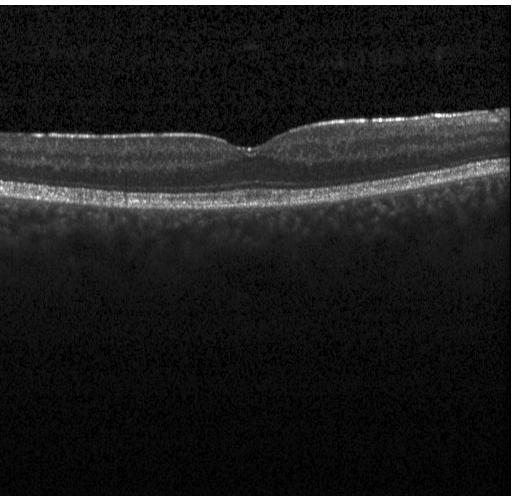

Assessment: no choroidal neovascularization, no diabetic macular edema, and no drusen.